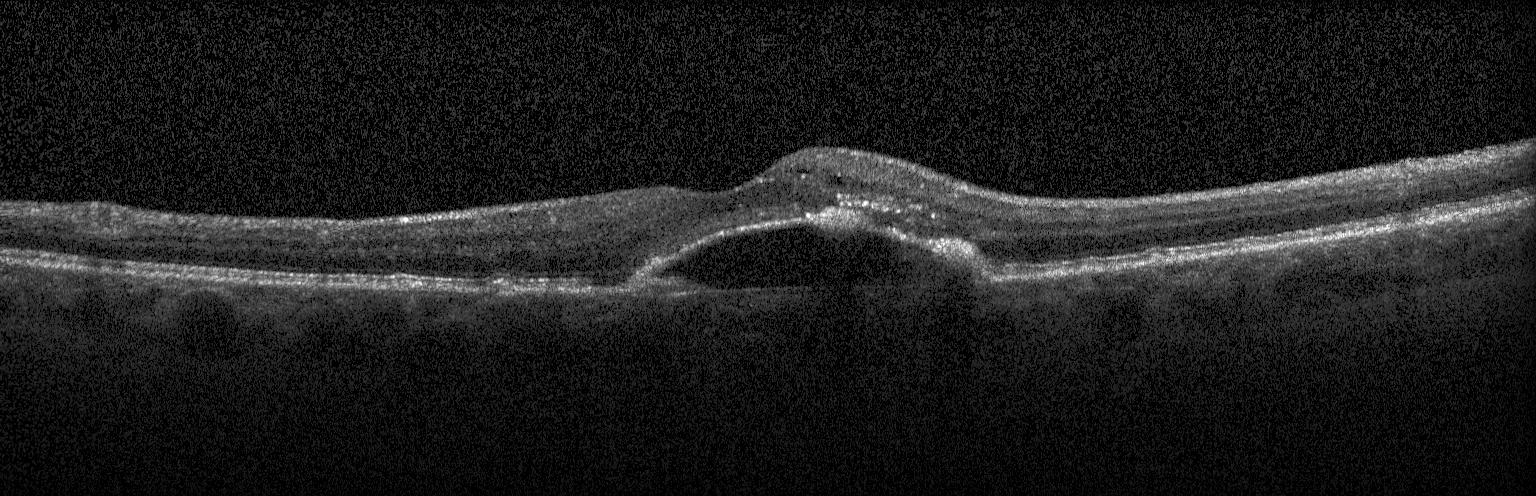
Impression: choroidal neovascularization (CNV).